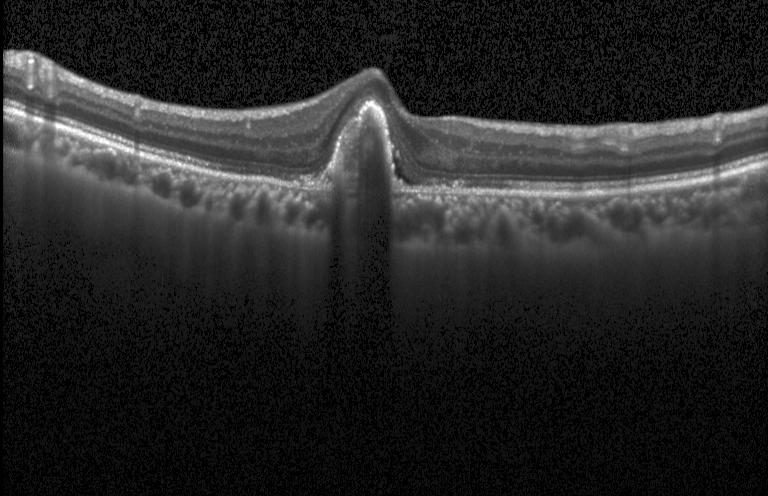

Spectral-domain optical coherence tomography, through the macula, OCT B-scan.
Finding: a choroidal neovascular membrane.